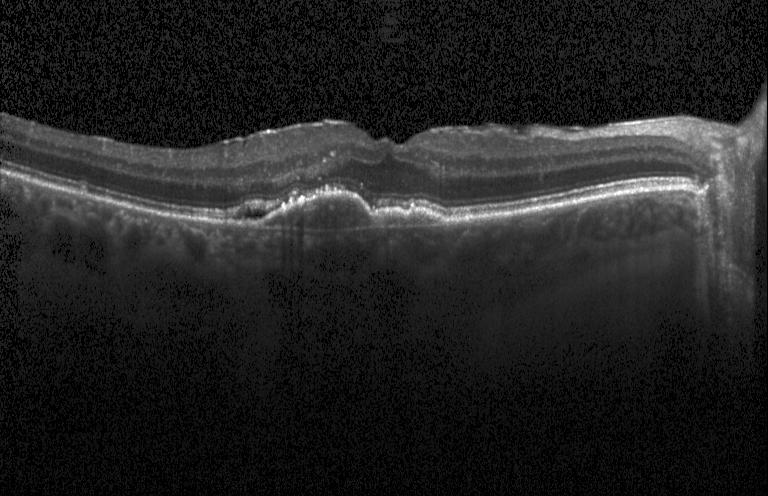 OCT B-scan. Spectral-domain OCT.
The scan shows a choroidal neovascular membrane.